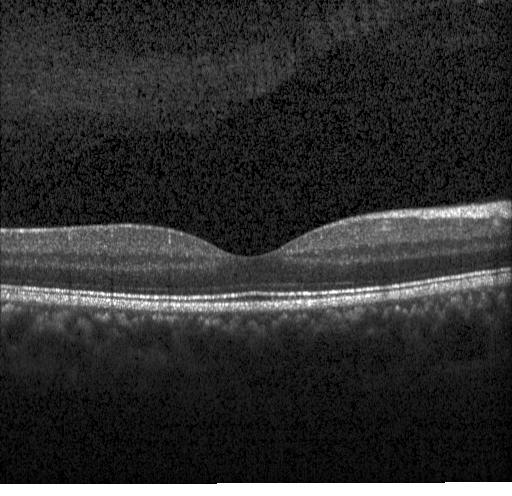 Instrument: Heidelberg Spectralis. Spectral-domain optical coherence tomography. Macular scan. OCT B-scan
Finding: no evidence of CNV, DME, or drusen.